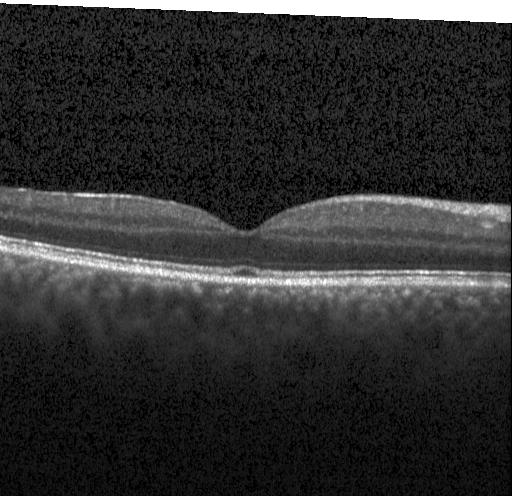 Horizontal scan through the fovea, spectral-domain OCT, Heidelberg Spectralis OCT system, retinal OCT B-scan. Finding: neither CNV, DME, nor drusen.